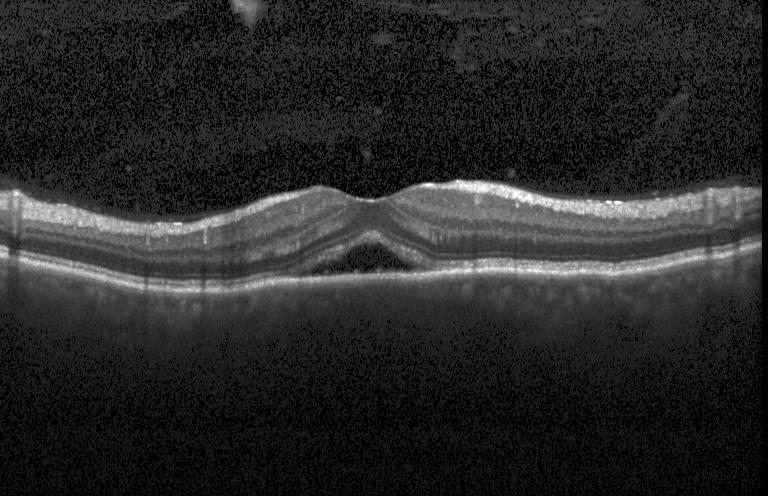

OCT line scan — Assessment: a choroidal neovascular membrane.